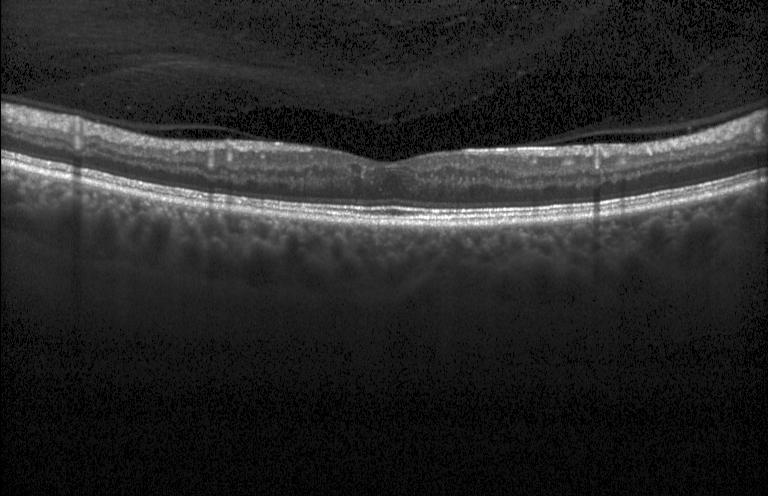

Spectral-domain optical coherence tomography, Heidelberg Spectralis OCT system, through the macula, OCT line scan.
Dx: no CNV, DME, or drusen.